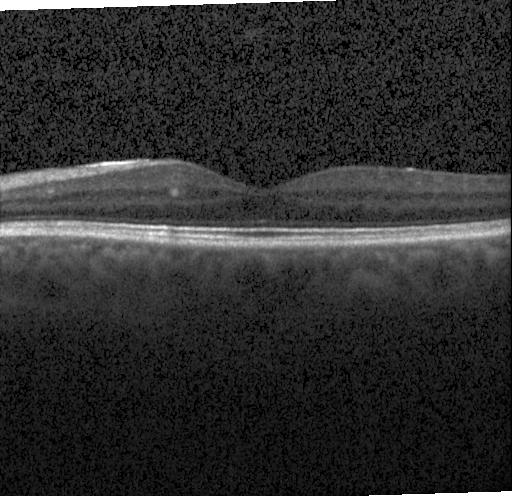
Instrument: Heidelberg Spectralis; optical coherence tomography scan.
Finding: no choroidal neovascularization, diabetic macular edema, or drusen.